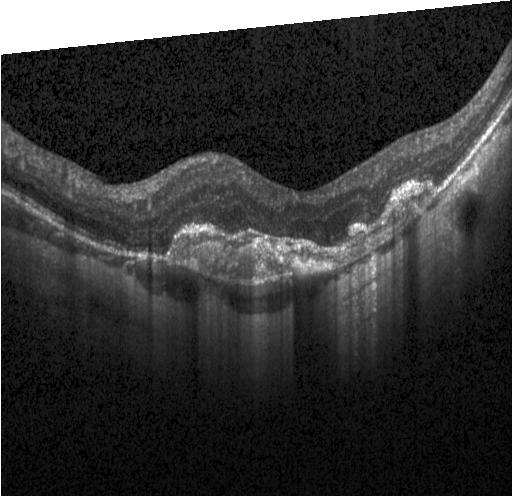

Assessment: a choroidal neovascular membrane.